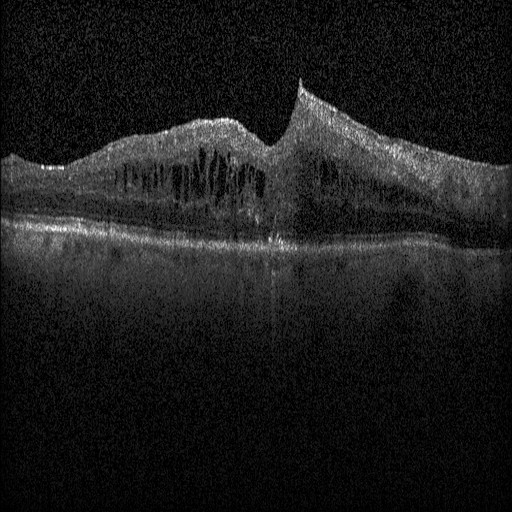 Diabetic macular edema (DME).